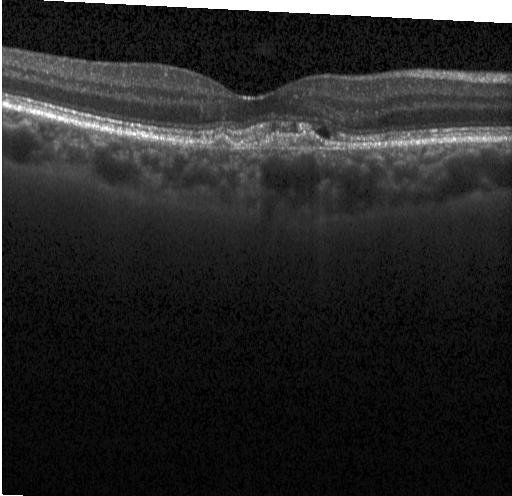 Diagnosis: a choroidal neovascular membrane.